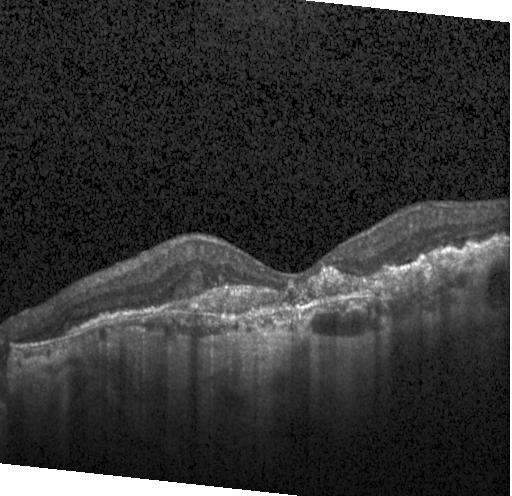 Heidelberg Spectralis, optical coherence tomography scan.
This B-scan demonstrates a choroidal neovascular membrane.